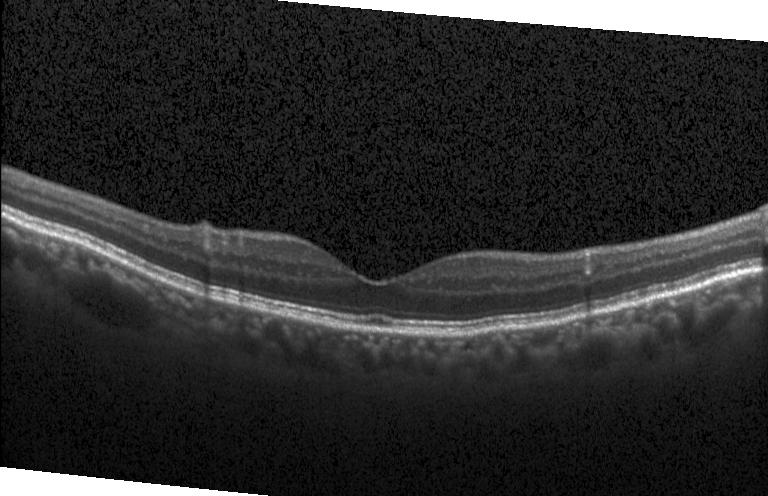 This B-scan demonstrates neither CNV, DME, nor drusen.